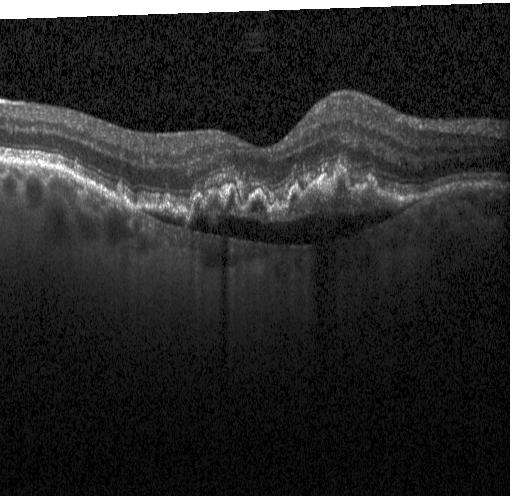

Through the macula; instrument: Heidelberg Spectralis; optical coherence tomography B-scan — OCT finding: a choroidal neovascular membrane.